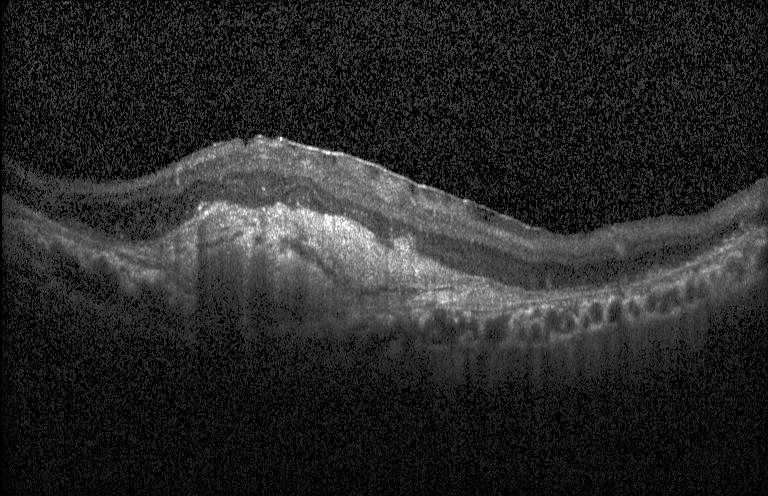

Retinal OCT cross-section.
Finding: choroidal neovascularization.